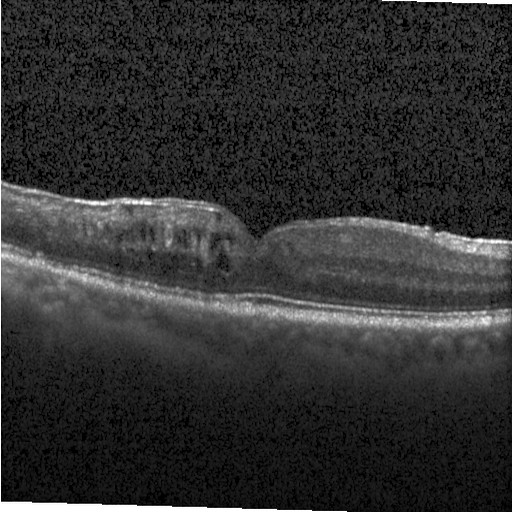

Diagnosis: diabetic macular edema.